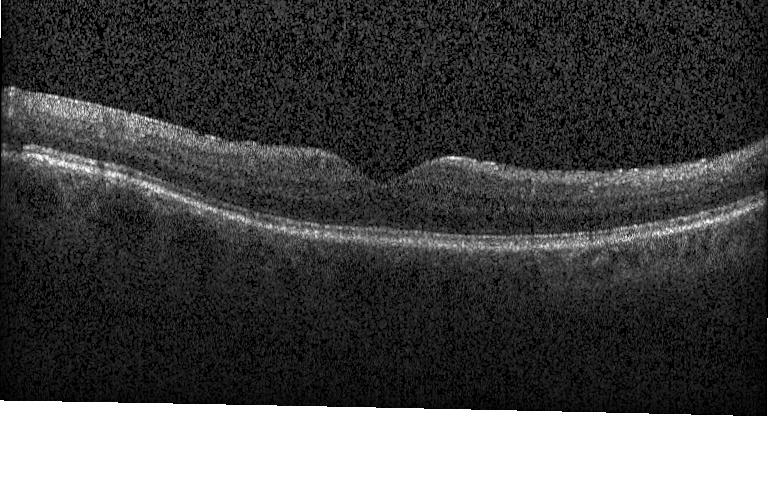
OCT B-scan, fovea-centered, spectral-domain OCT — Finding: no choroidal neovascularization, diabetic macular edema, or drusen.